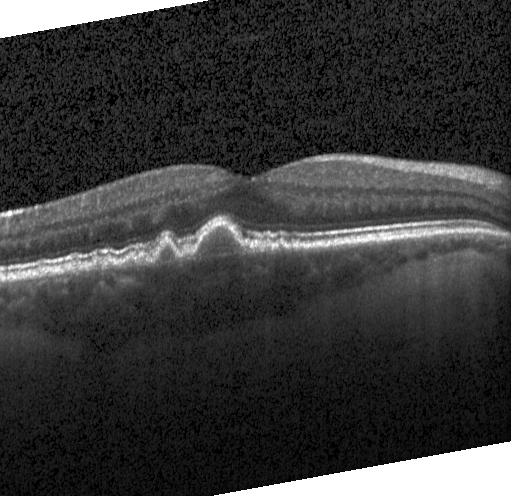

Macular OCT demonstrating multiple drusen.